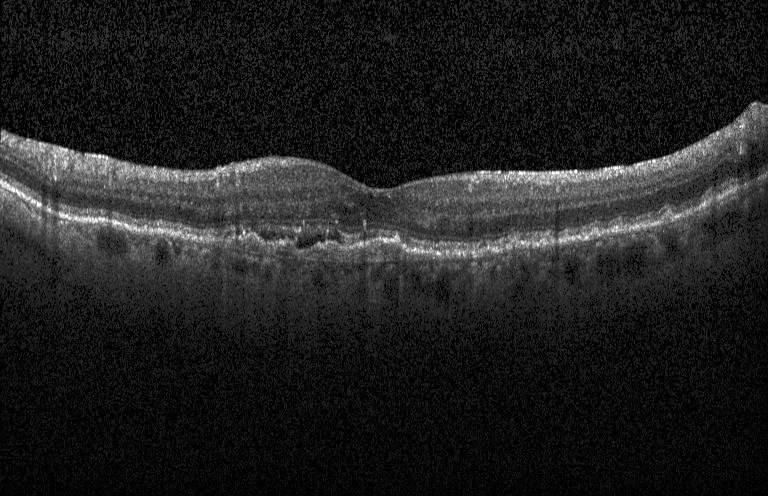 OCT finding: choroidal neovascularization (CNV).